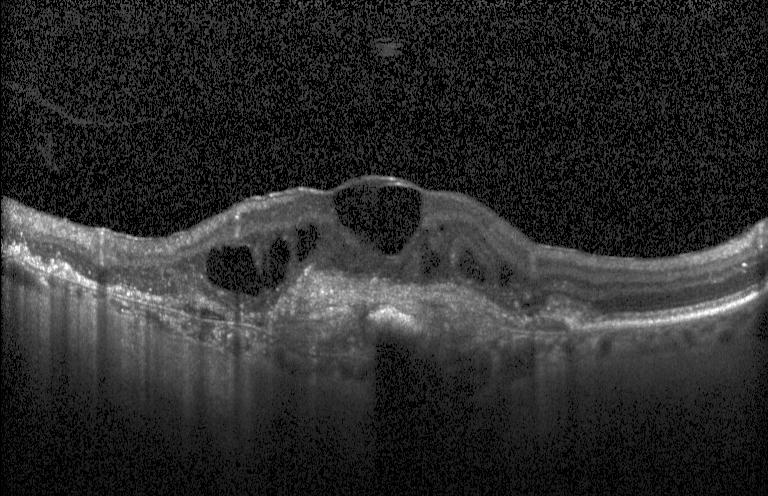

Retinal OCT cross-section — Impression: a choroidal neovascular membrane.